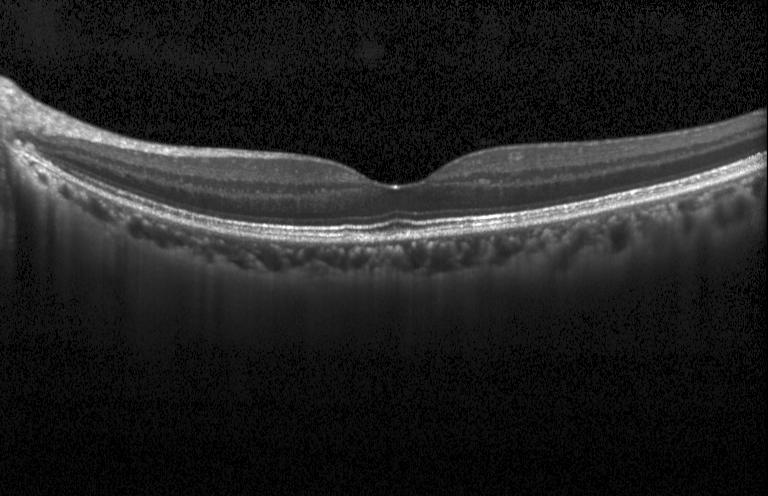

Optical coherence tomography B-scan, spectral-domain optical coherence tomography, Heidelberg Spectralis — Macular OCT: no choroidal neovascularization, diabetic macular edema, or drusen.